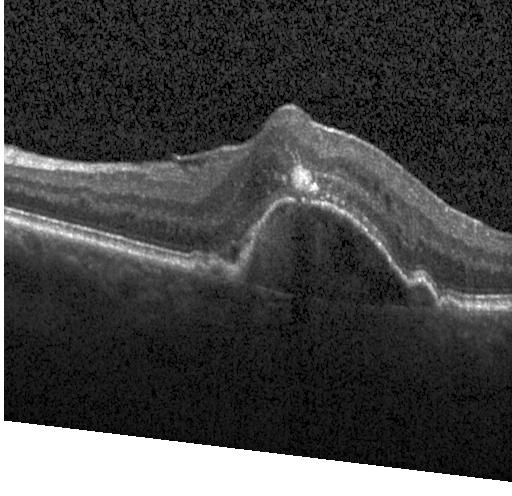 Retinal OCT B-scan. Instrument: Heidelberg Spectralis. SD-OCT. Centered on the fovea. Finding: a choroidal neovascular membrane.